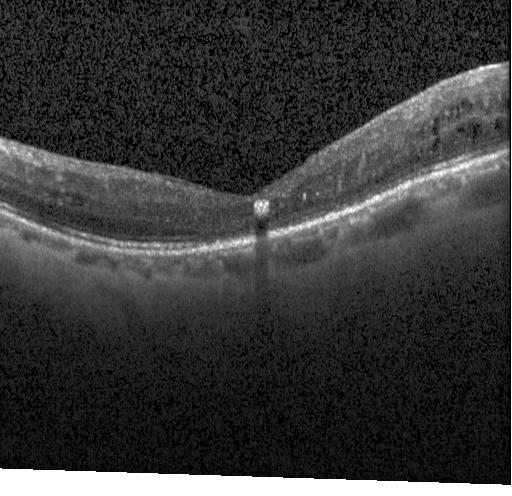

Impression: DME.